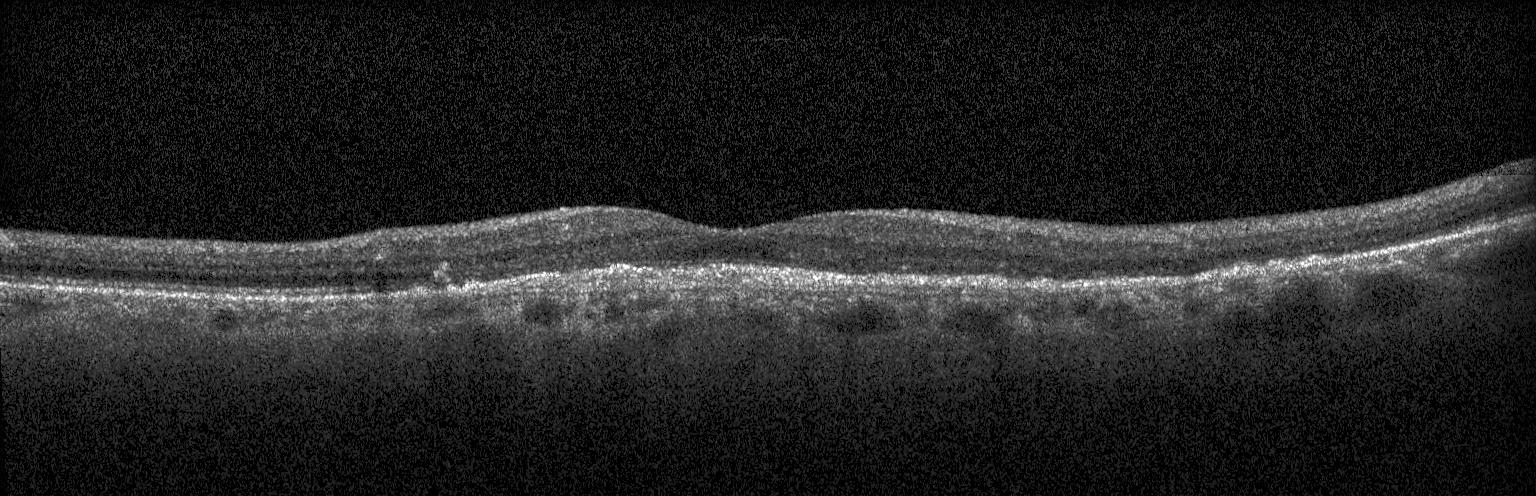

Horizontal scan through the fovea. Optical coherence tomography scan. Spectral-domain OCT. Instrument: Heidelberg Spectralis
Impression: a choroidal neovascular membrane.